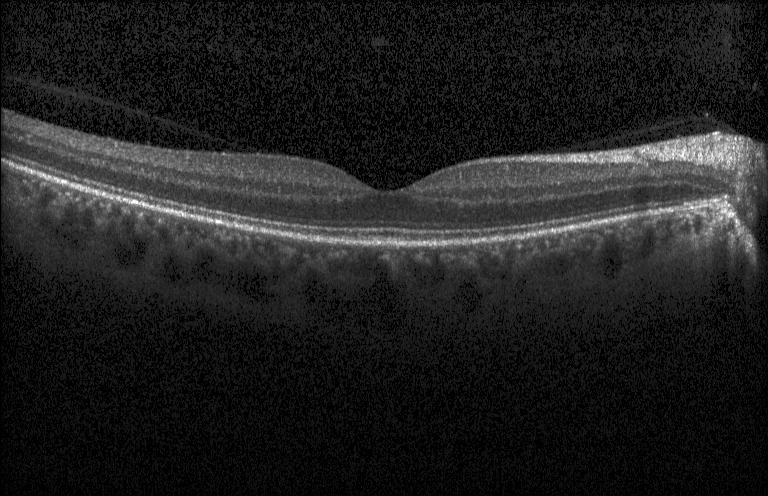
Spectral-domain OCT; optical coherence tomography B-scan. Impression: no evidence of CNV, DME, or drusen.